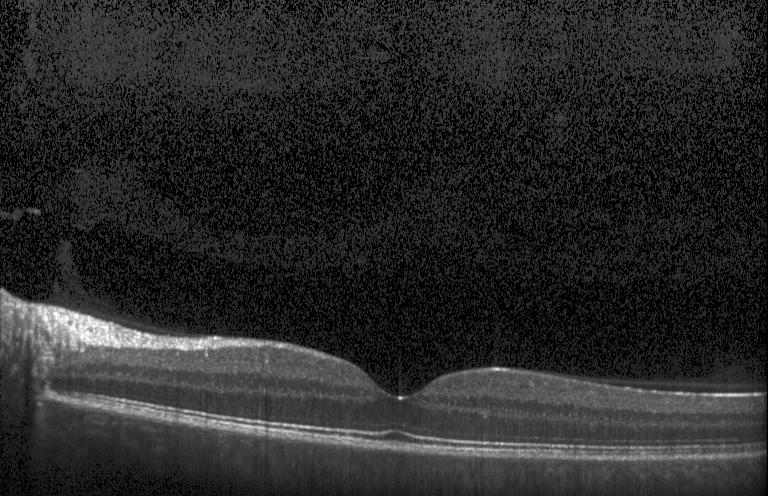

Spectral-domain OCT B-scan: no evidence of CNV, DME, or drusen.